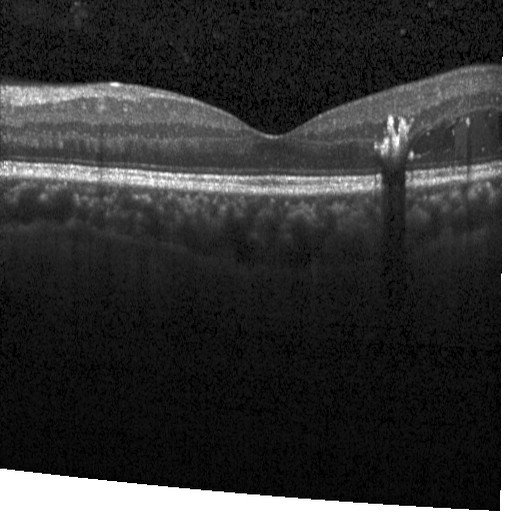
Retinal OCT B-scan
Diabetic macular edema.